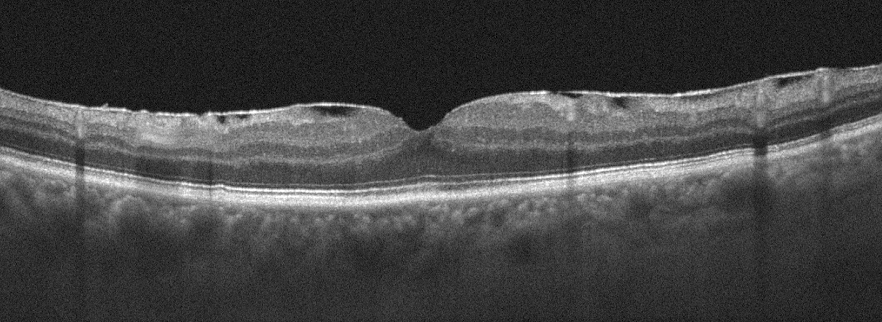

Oculus dexter · optical coherence tomography B-scan · macular scan
Finding: epiretinal membrane (ERM).